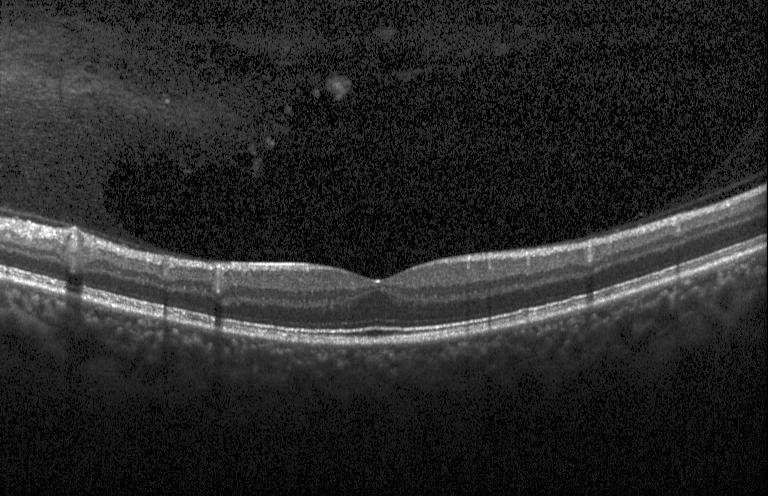

Diagnosis: no choroidal neovascularization, no diabetic macular edema, and no drusen.